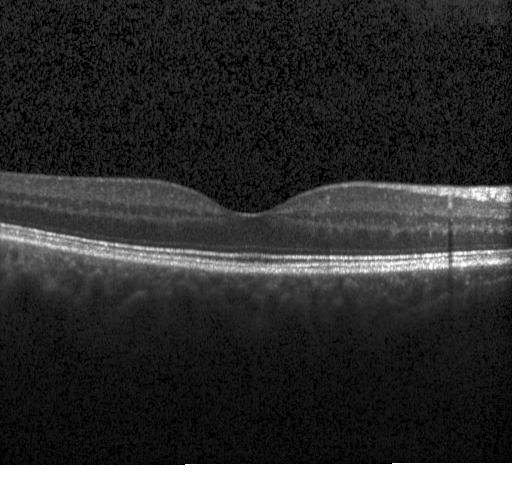

Spectral-domain OCT · horizontal scan through the fovea · OCT line scan.
Assessment: no evidence of choroidal neovascularization, diabetic macular edema, or drusen.